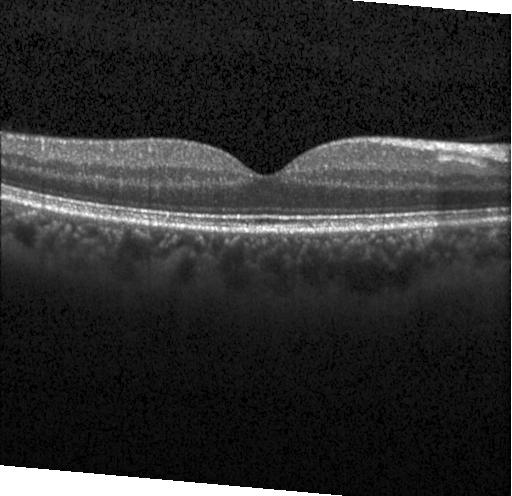 OCT B-scan showing neither CNV, DME, nor drusen.